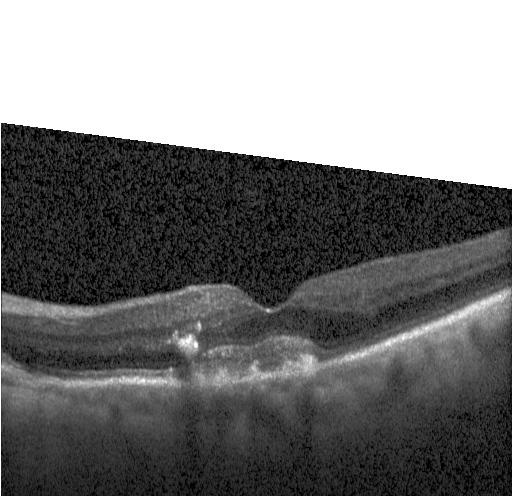
Optical coherence tomography scan. SD-OCT — Assessment: choroidal neovascularization (CNV).